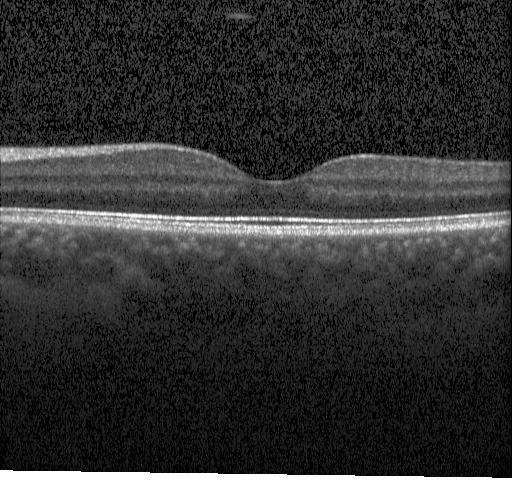 Spectral-domain optical coherence tomography, fovea-centered, retinal OCT cross-section
The scan shows no choroidal neovascularization, no diabetic macular edema, and no drusen.